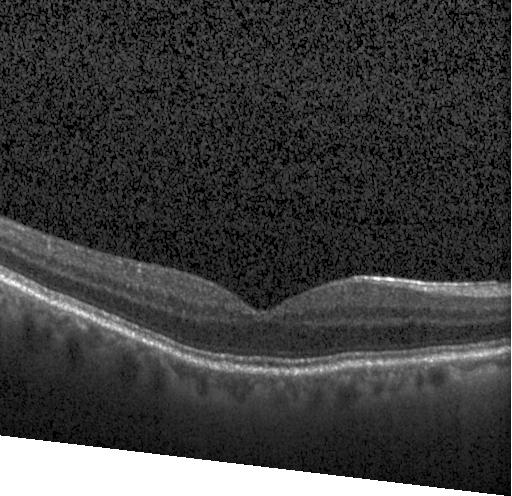
Spectral-domain OCT B-scan: neither choroidal neovascularization, diabetic macular edema, nor drusen.